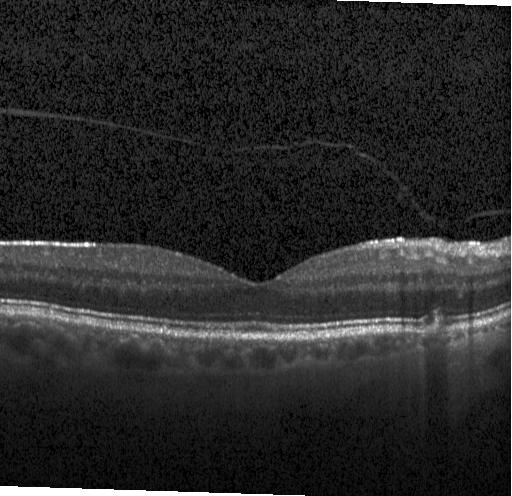
Diagnosis: drusen.